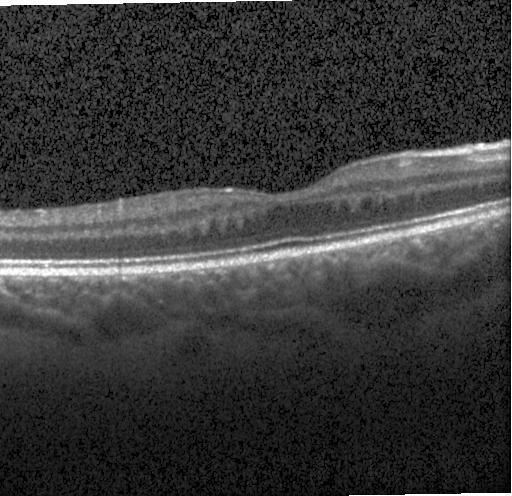
Optical coherence tomography B-scan. Acquired on a Heidelberg Spectralis. Spectral-domain optical coherence tomography
Dx: no CNV, no DME, and no drusen.